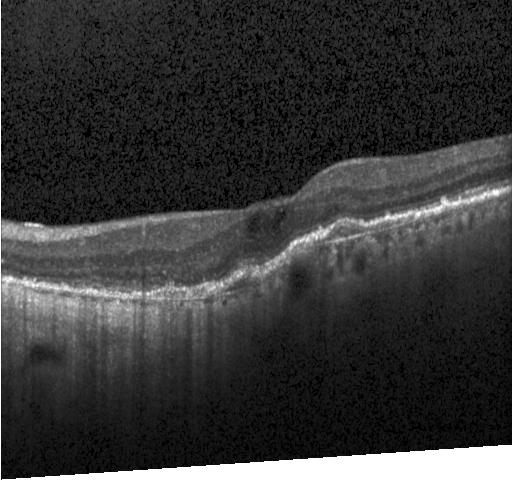

Diagnosis: a choroidal neovascular membrane.